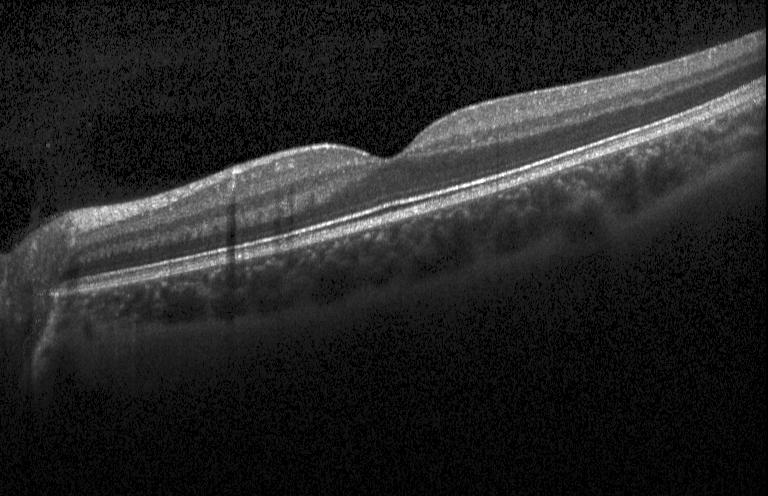 Diagnosis: neither choroidal neovascularization, diabetic macular edema, nor drusen.